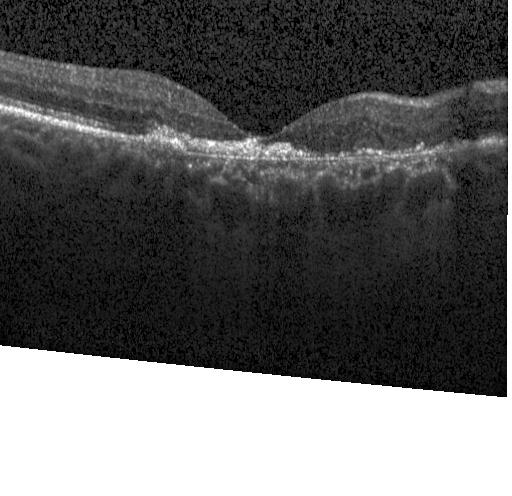
Assessment: a choroidal neovascular membrane.